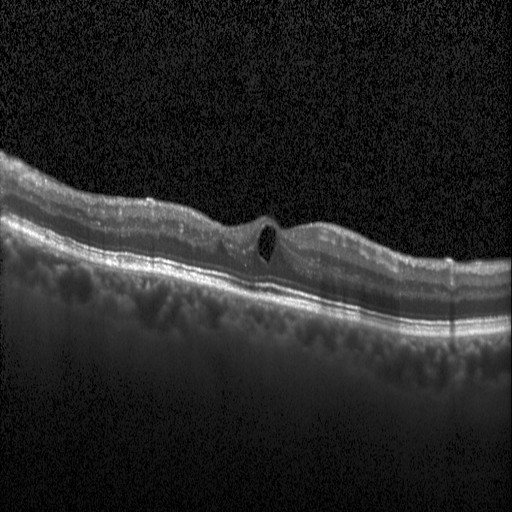

Finding: diabetic macular edema (DME).